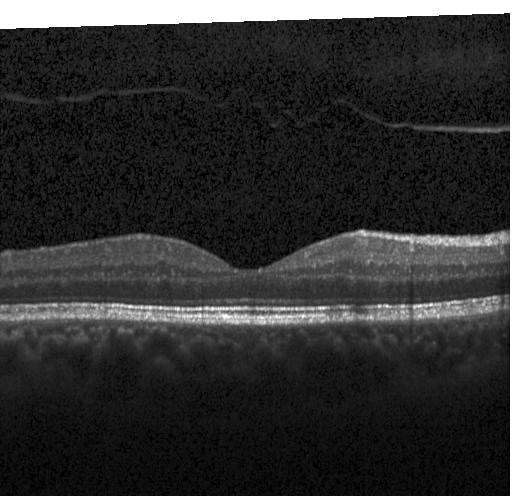

Centered on the fovea · optical coherence tomography B-scan · SD-OCT
Assessment: no choroidal neovascularization, no diabetic macular edema, and no drusen.